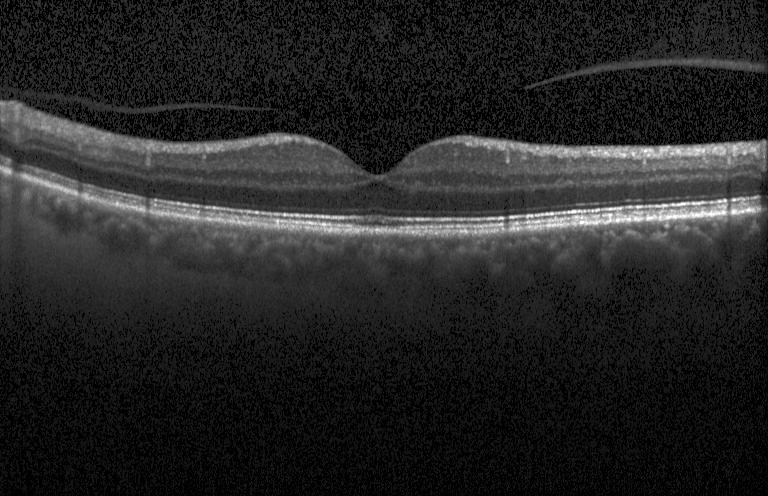
Macular scan; retinal OCT B-scan. Impression: no choroidal neovascularization, no diabetic macular edema, and no drusen.